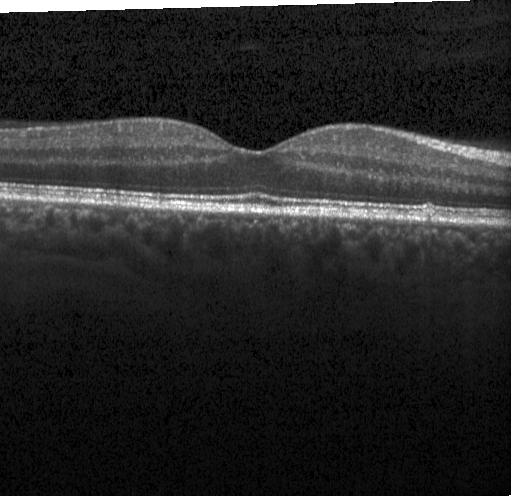
OCT scan showing no choroidal neovascularization, diabetic macular edema, or drusen.